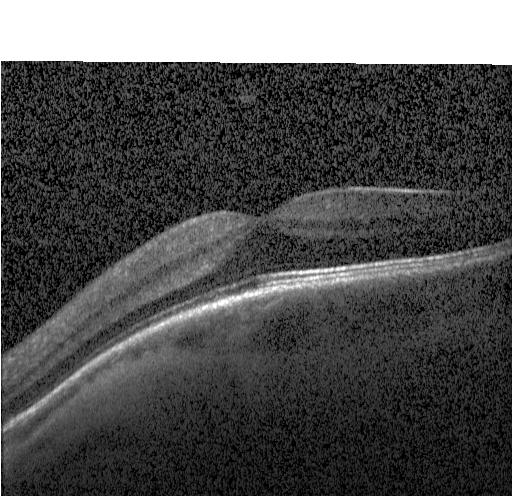 Spectral-domain optical coherence tomography. OCT line scan. Assessment: no evidence of CNV, DME, or drusen.